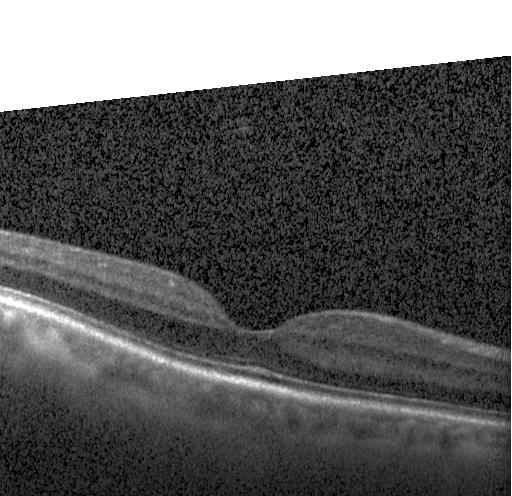

OCT B-scan
Neither choroidal neovascularization, diabetic macular edema, nor drusen.